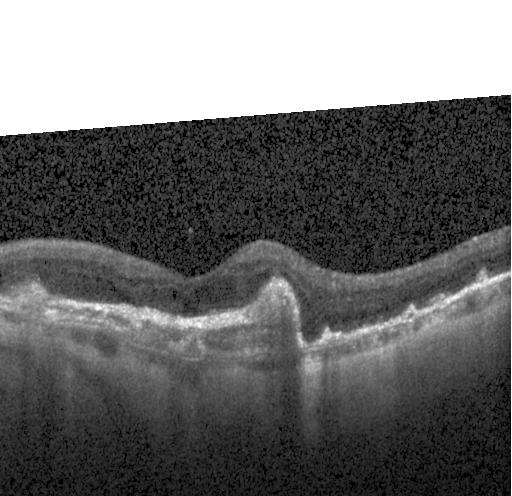

Diagnosis: a choroidal neovascular membrane.